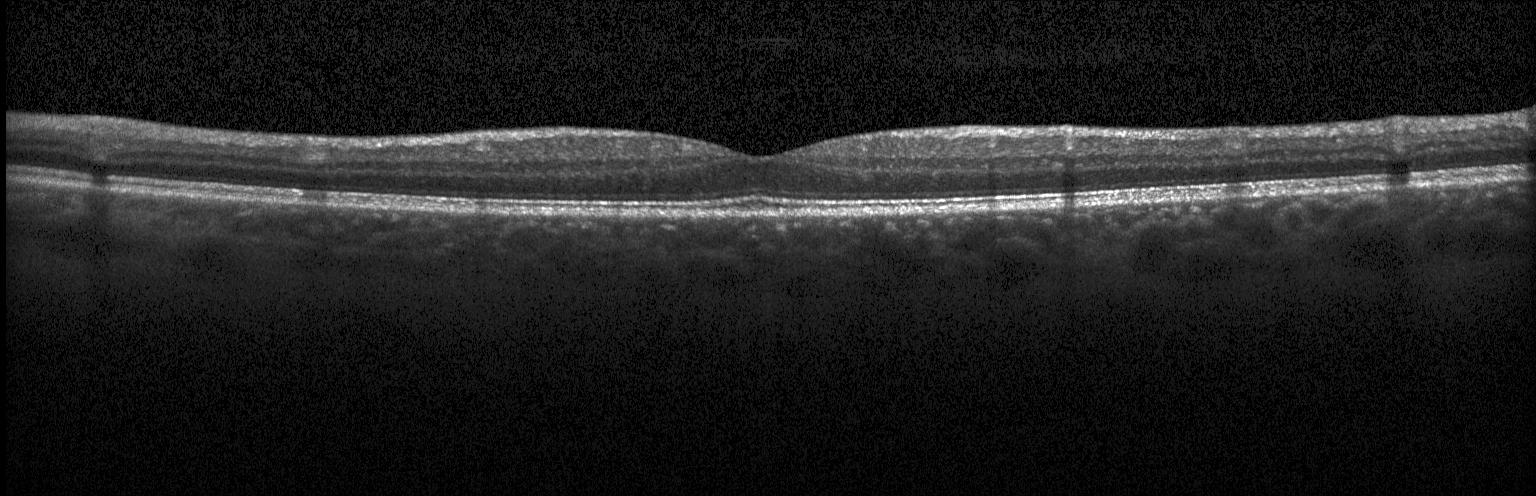
Instrument: Heidelberg Spectralis, through the macula, retinal OCT B-scan
Impression: neither CNV, DME, nor drusen.